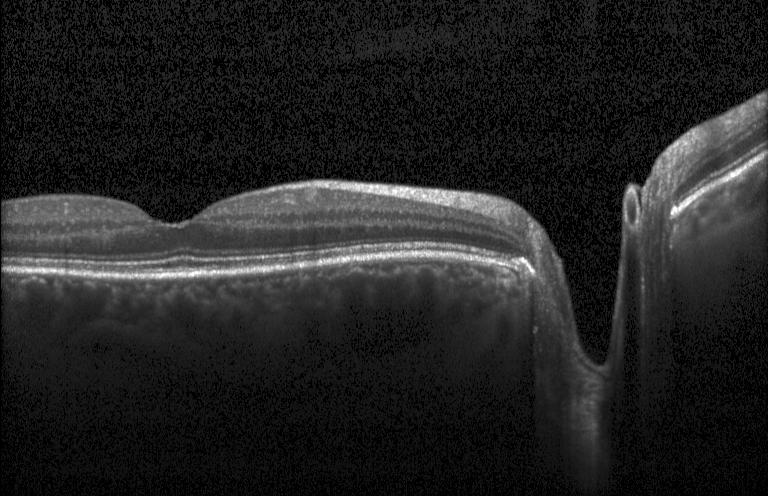 Retinal OCT B-scan — Finding: neither choroidal neovascularization, diabetic macular edema, nor drusen.